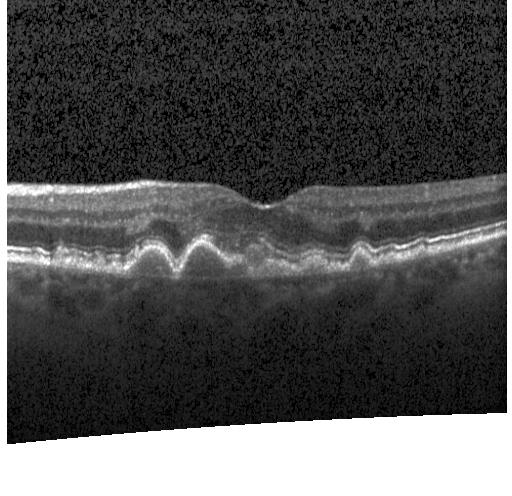 This B-scan demonstrates a choroidal neovascular membrane.